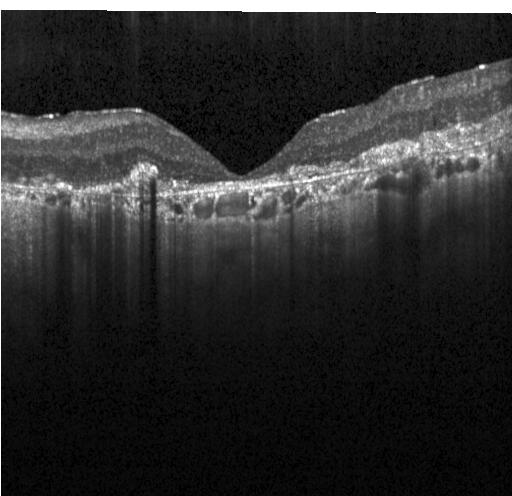 SD-OCT · instrument: Heidelberg Spectralis · optical coherence tomography B-scan · centered on the fovea. Dx: a choroidal neovascular membrane.